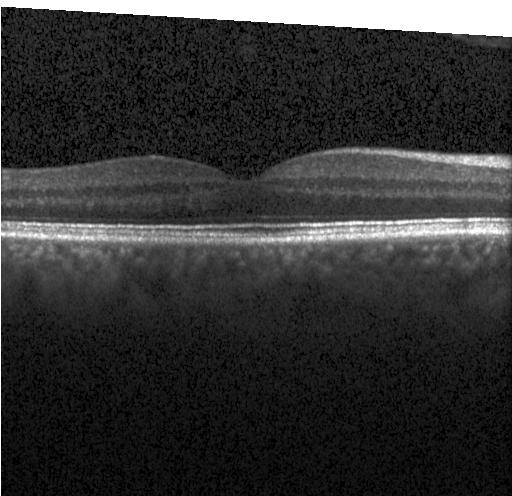

Dx: no evidence of choroidal neovascularization, diabetic macular edema, or drusen.